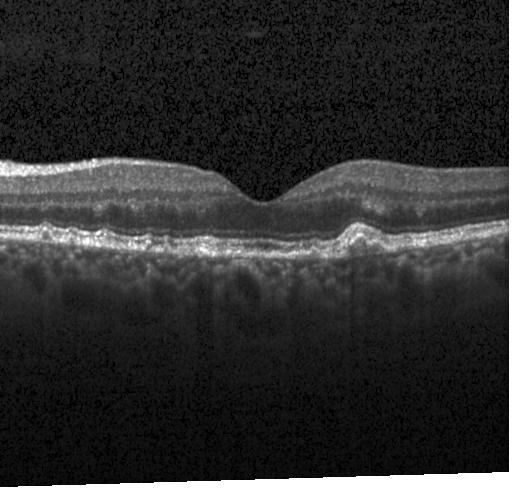

Diagnosis: multiple drusen.